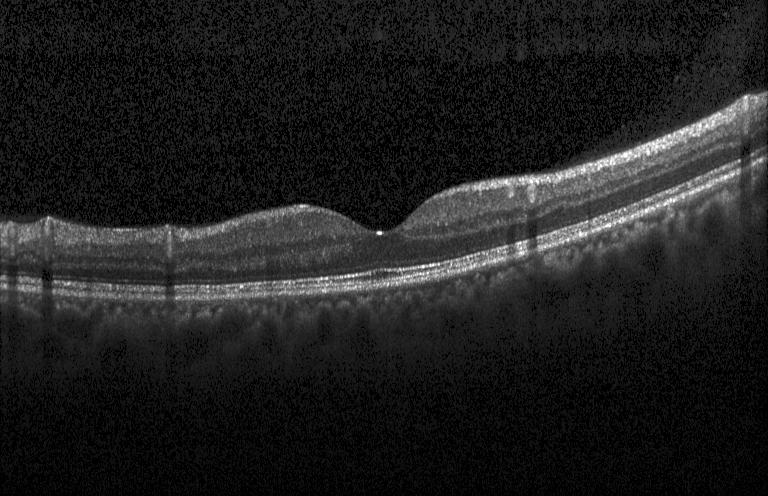
Retinal OCT cross-section
No evidence of choroidal neovascularization, diabetic macular edema, or drusen.